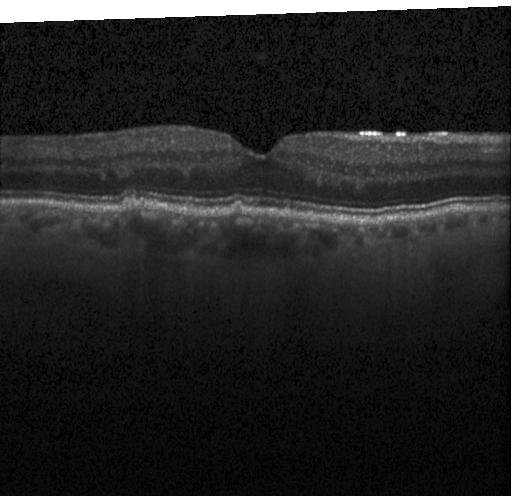

Heidelberg Spectralis OCT system. Spectral-domain optical coherence tomography. Retinal OCT B-scan. Fovea-centered. Macular OCT: multiple drusen.